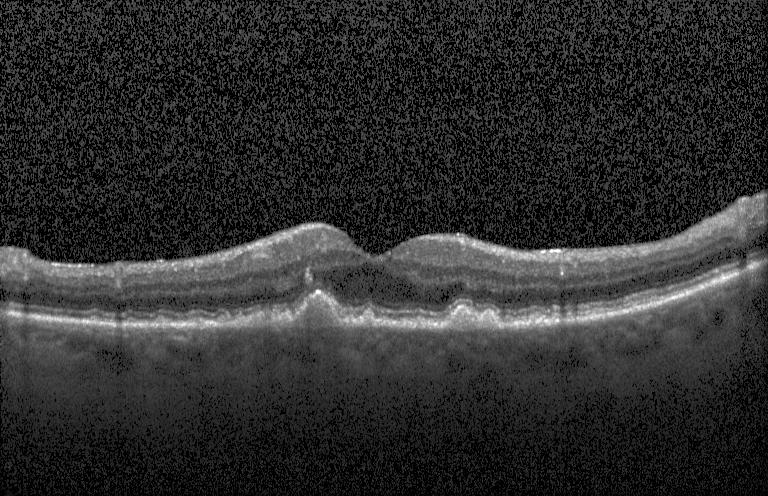 Spectral-domain optical coherence tomography. OCT line scan. Acquired on a Heidelberg Spectralis. Horizontal scan through the fovea
The scan shows sub-RPE drusenoid deposits.